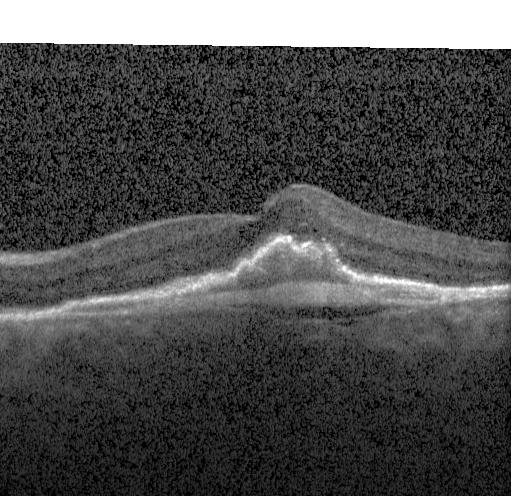 This B-scan demonstrates choroidal neovascularization.